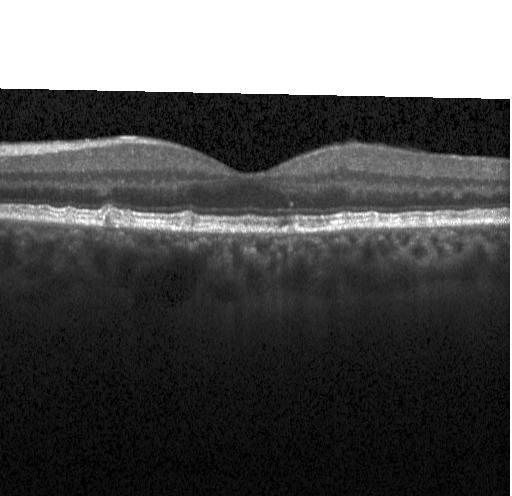

OCT B-scan. Dx: multiple drusen.